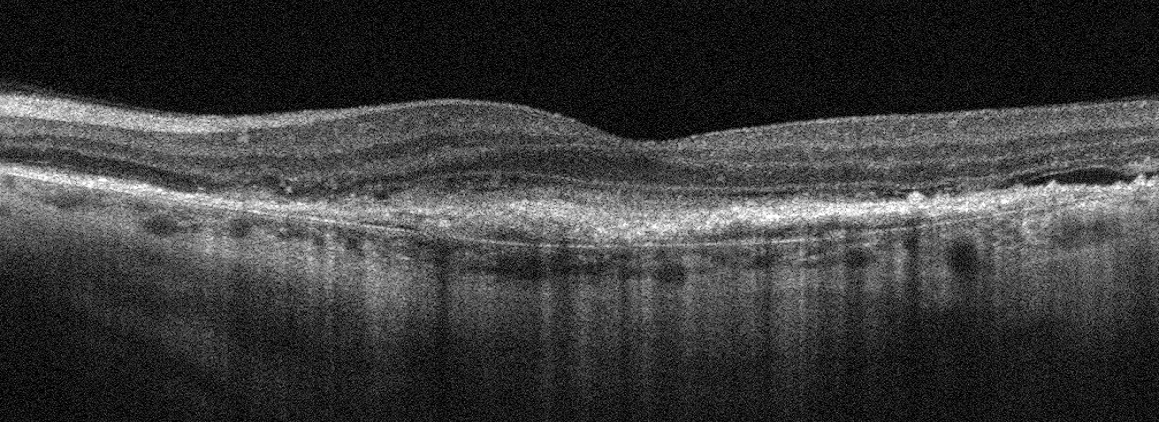

Fovea-centered; left eye; optical coherence tomography scan; acquired on an Optovue Avanti RTVue XR.
Finding: AMD.